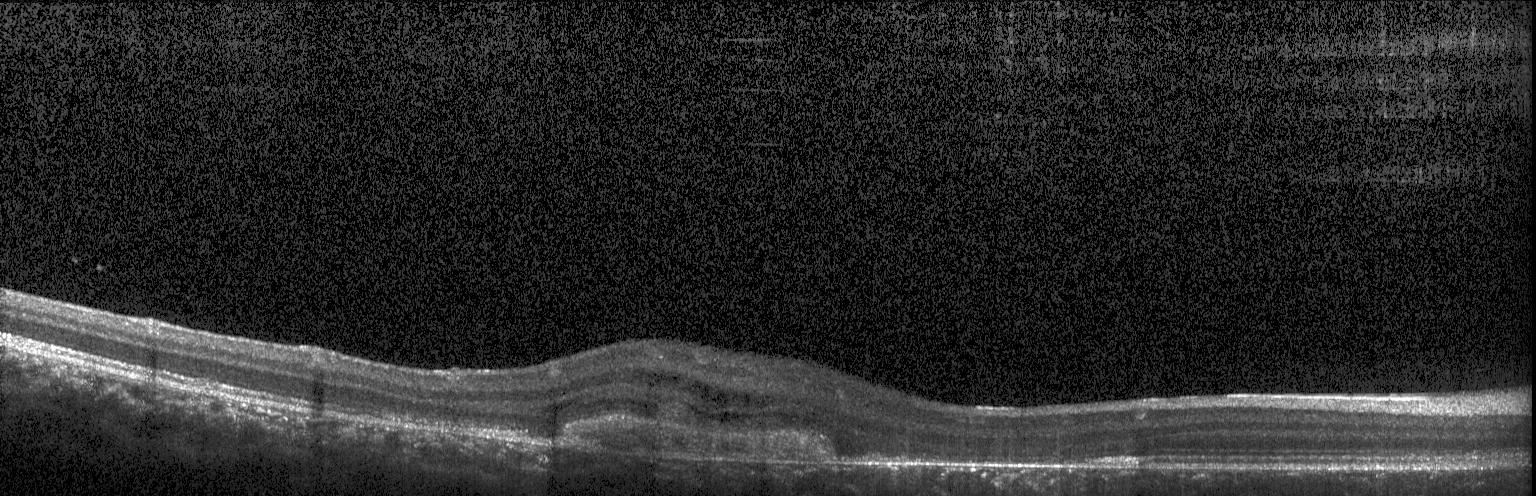 OCT line scan
Impression: CNV.